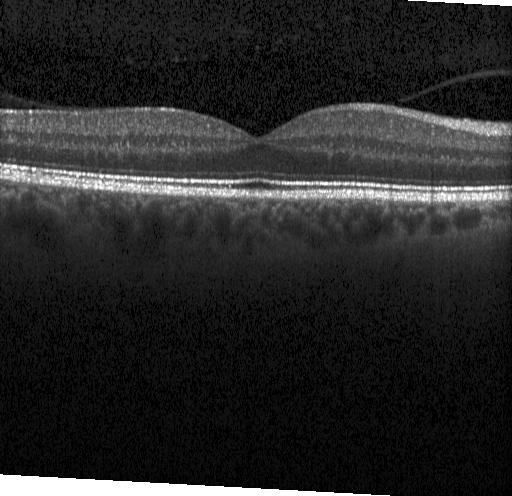 Macular OCT: neither choroidal neovascularization, diabetic macular edema, nor drusen.